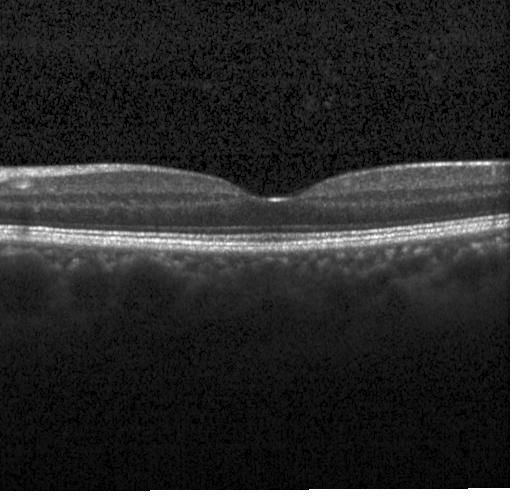
Macular OCT: no CNV, no DME, and no drusen.